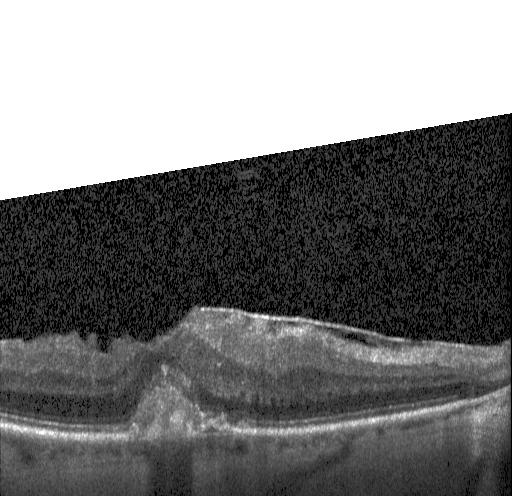 Diagnosis: CNV.